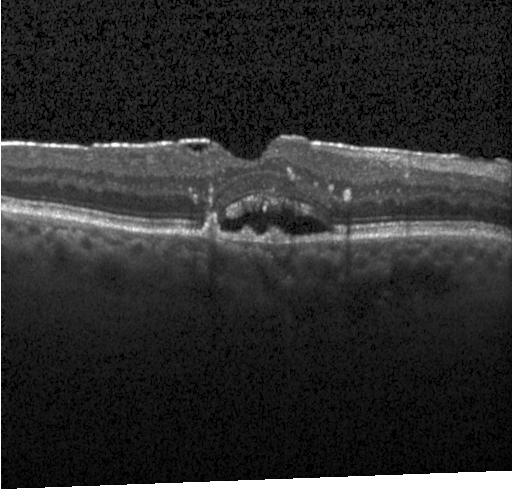 Retinal OCT B-scan; Heidelberg Spectralis
OCT finding: choroidal neovascularization.